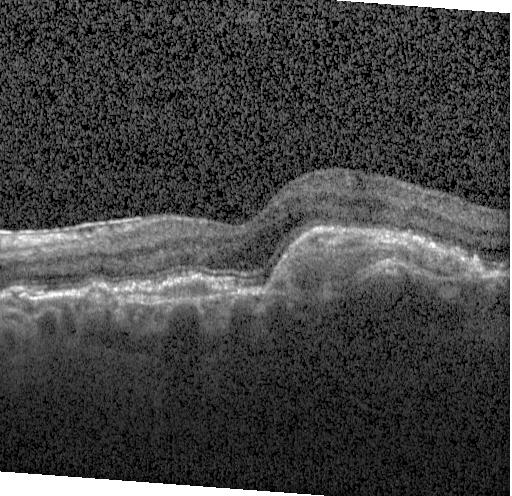
SD-OCT, OCT line scan.
Finding: choroidal neovascularization.